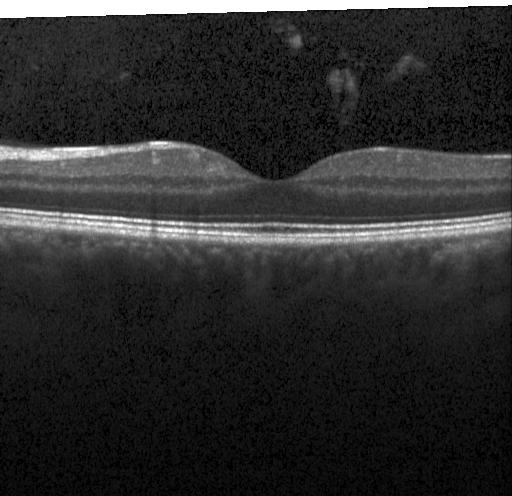
OCT B-scan.
Finding: neither choroidal neovascularization, diabetic macular edema, nor drusen.